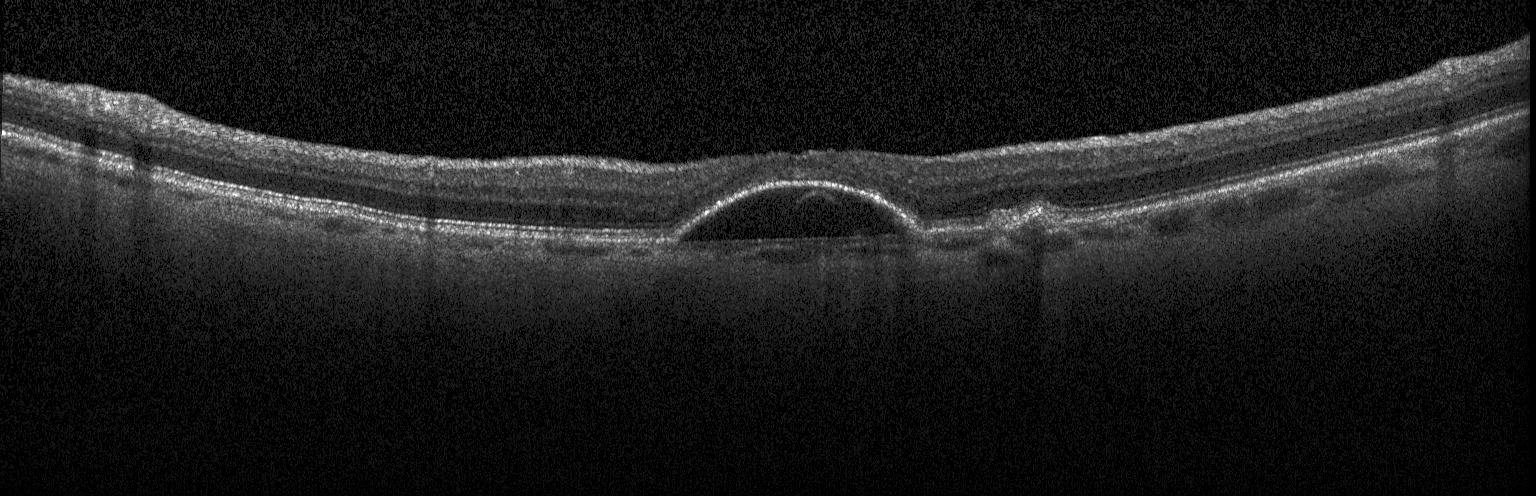 OCT finding: a choroidal neovascular membrane.